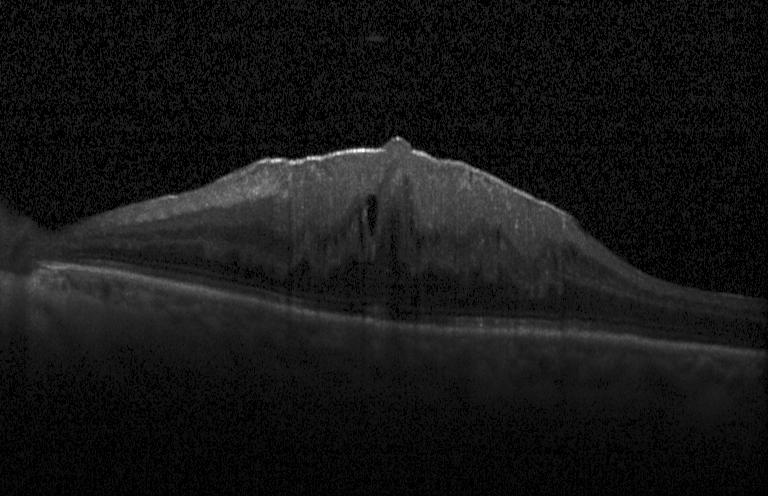 Fovea-centered · optical coherence tomography B-scan · spectral-domain OCT. Assessment: DME.